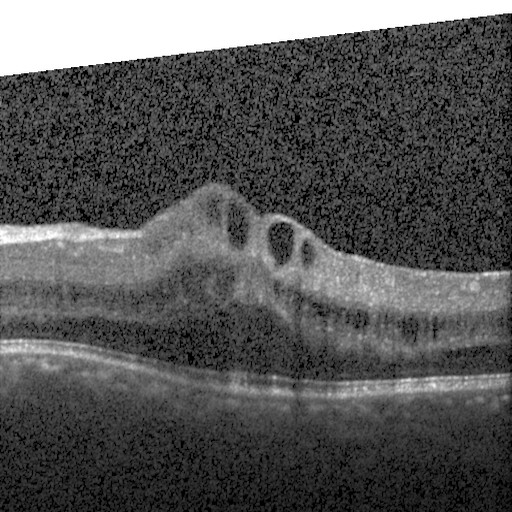

Heidelberg Spectralis. Optical coherence tomography scan — Impression: DME.